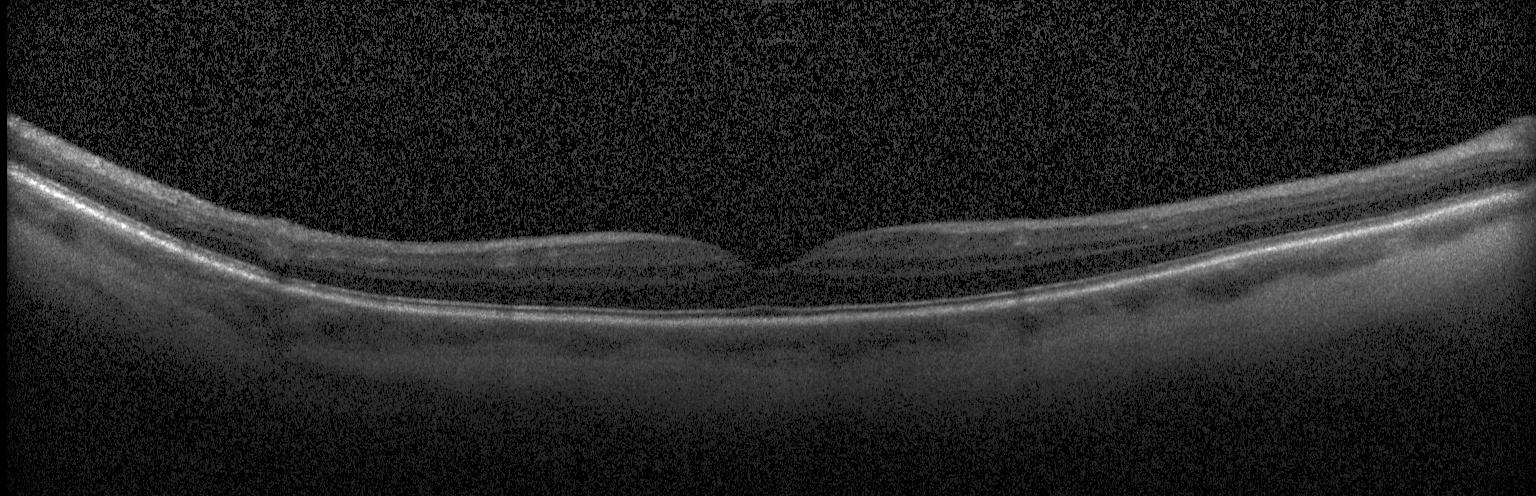
Retinal OCT B-scan; acquired on a Heidelberg Spectralis
Assessment: no evidence of CNV, DME, or drusen.